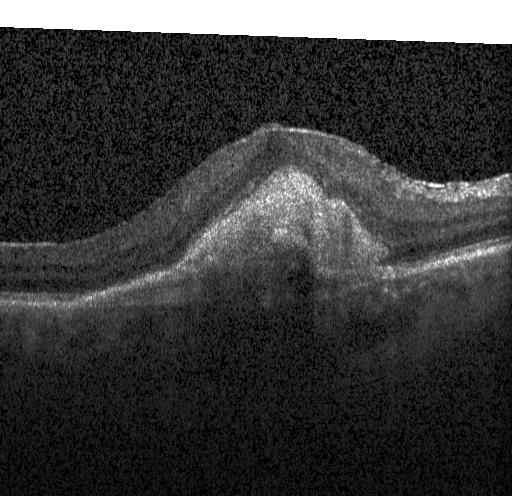
OCT B-scan; acquired on a Heidelberg Spectralis; SD-OCT — Impression: a choroidal neovascular membrane.